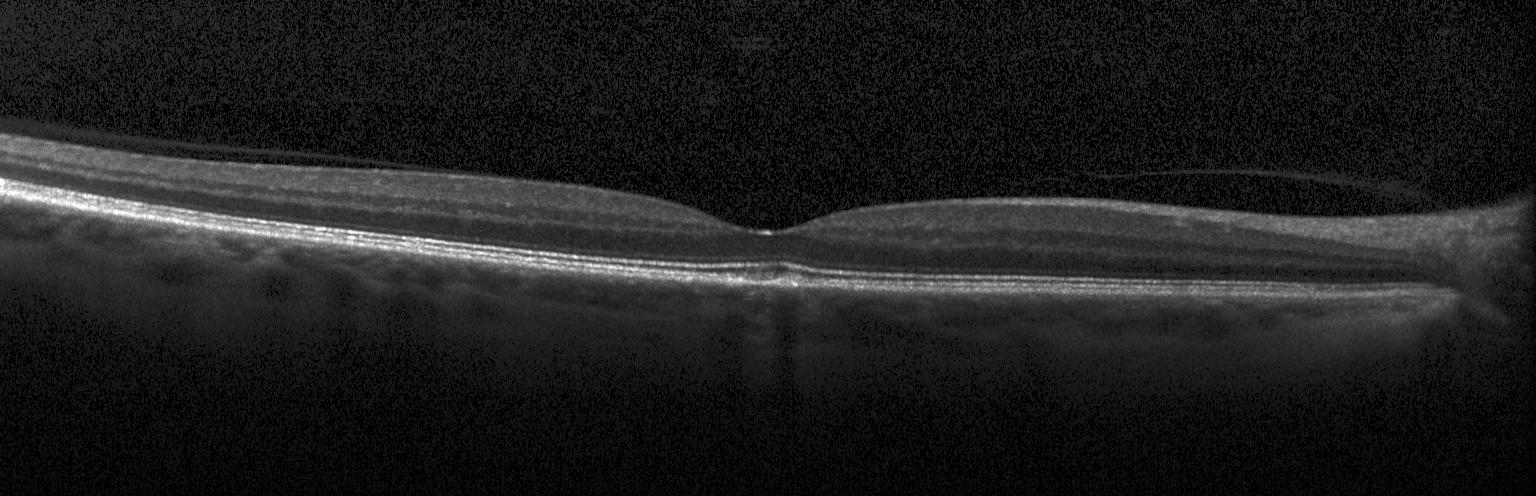

Diagnosis: no choroidal neovascularization, diabetic macular edema, or drusen.